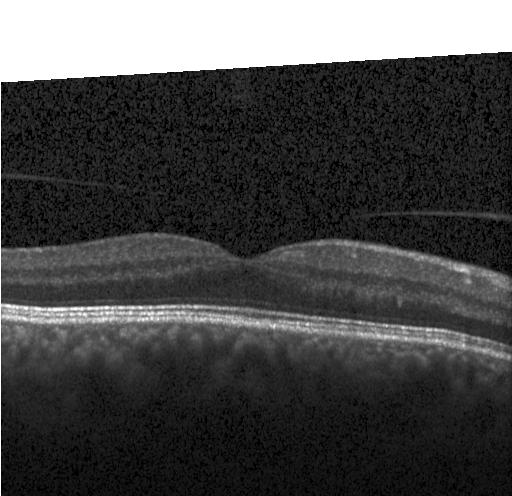 Dx: no evidence of choroidal neovascularization, diabetic macular edema, or drusen.